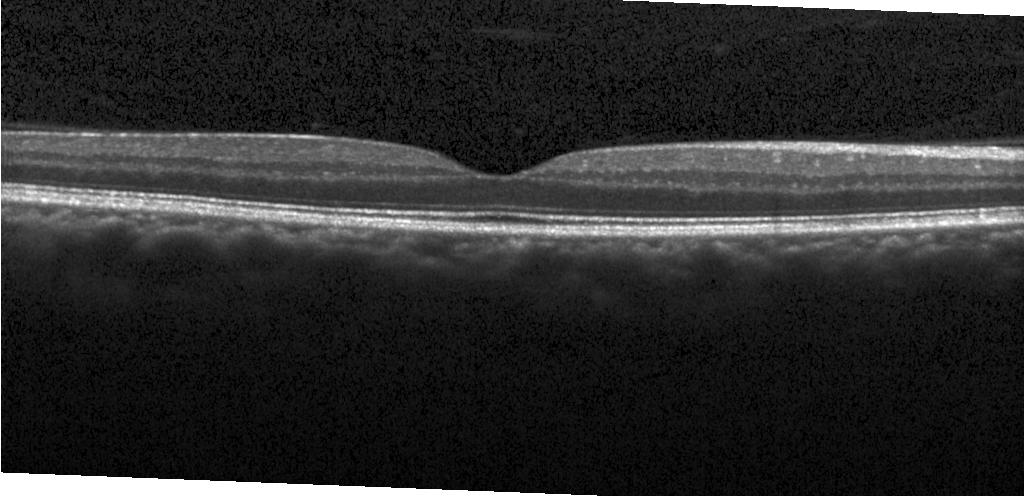

Finding: no CNV, DME, or drusen.